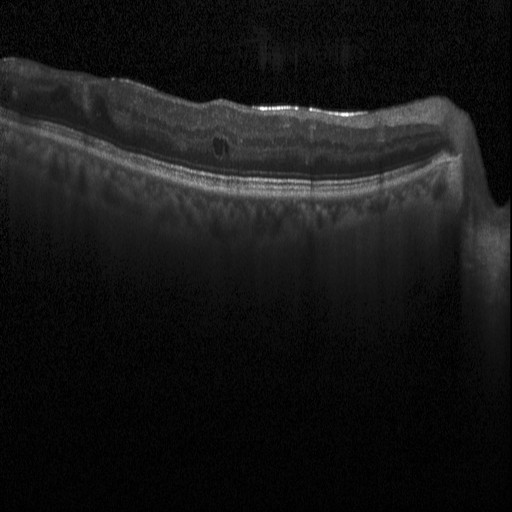 Spectral-domain optical coherence tomography · optical coherence tomography scan — Dx: diabetic macular edema (DME).